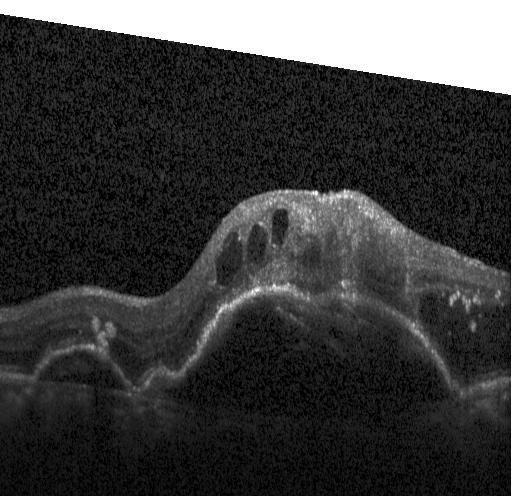

OCT finding: a choroidal neovascular membrane.